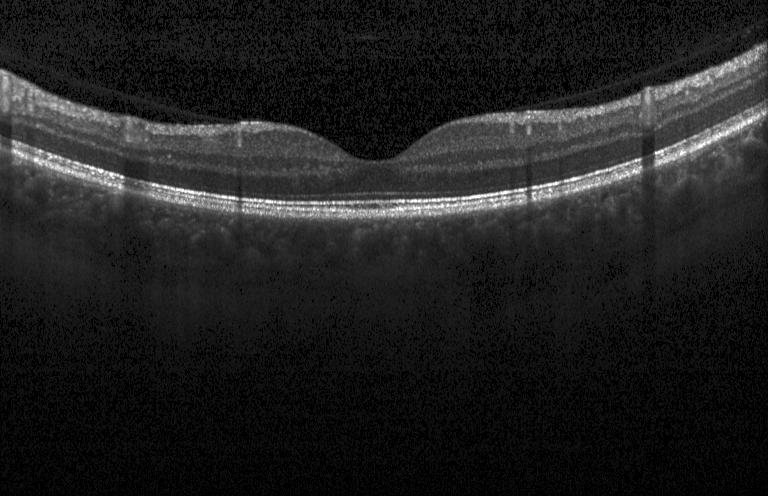

No choroidal neovascularization, no diabetic macular edema, and no drusen.